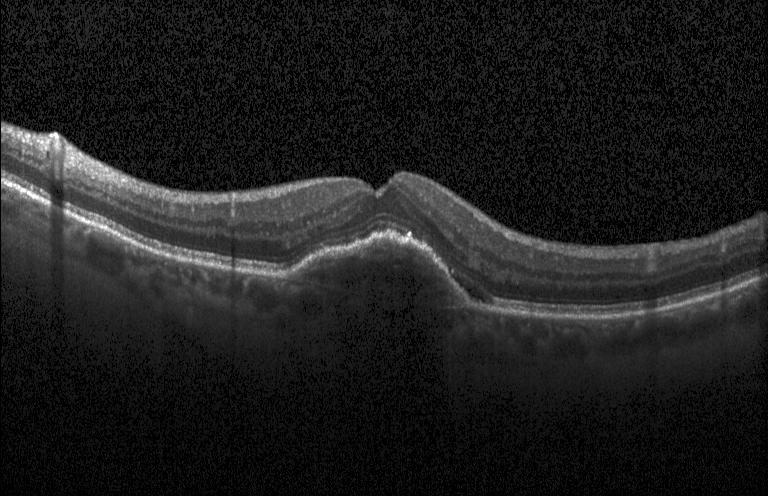
Retinal OCT cross-section.
This B-scan demonstrates a choroidal neovascular membrane.